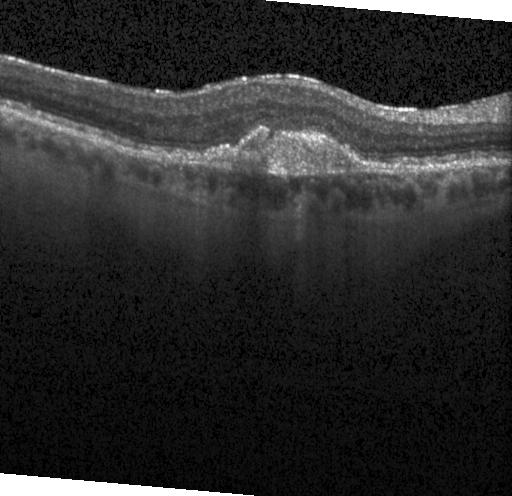
Diagnosis: a choroidal neovascular membrane.